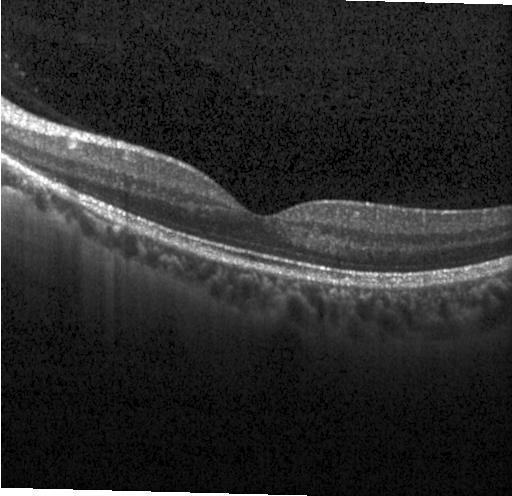

OCT line scan, acquired on a Heidelberg Spectralis. Assessment: no choroidal neovascularization, diabetic macular edema, or drusen.